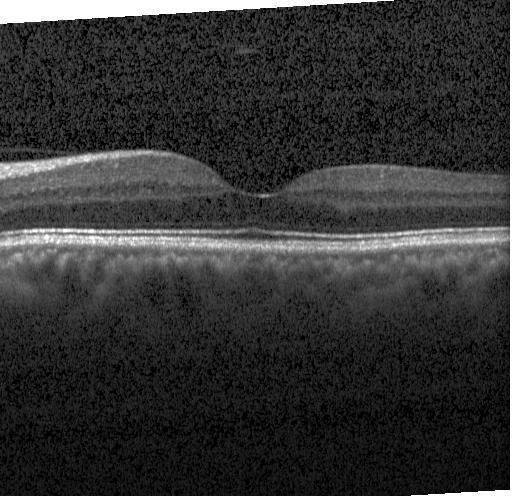
Heidelberg Spectralis OCT system. Retinal OCT B-scan. Spectral-domain optical coherence tomography. Fovea-centered — Impression: no evidence of CNV, DME, or drusen.